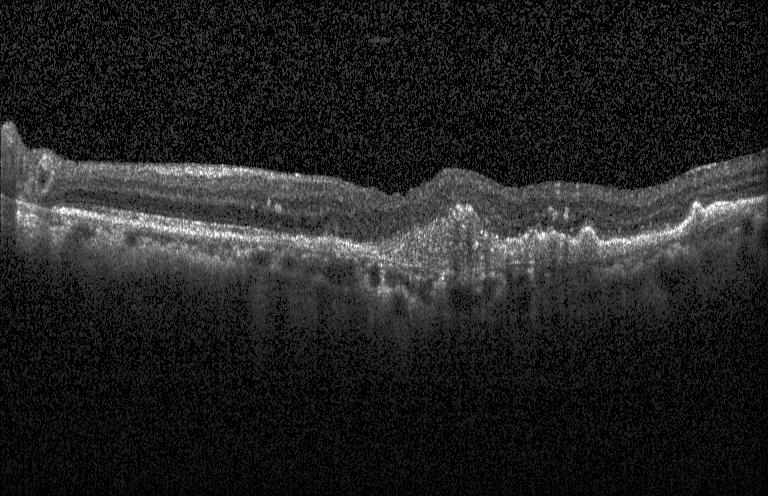
Retinal OCT cross-section. Spectral-domain optical coherence tomography. A choroidal neovascular membrane.